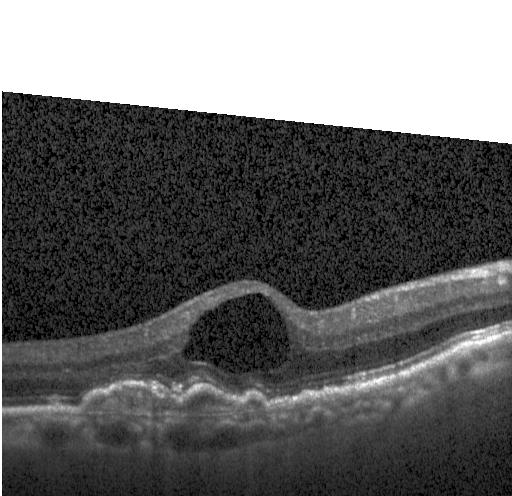 OCT B-scan — Finding: choroidal neovascularization (CNV).